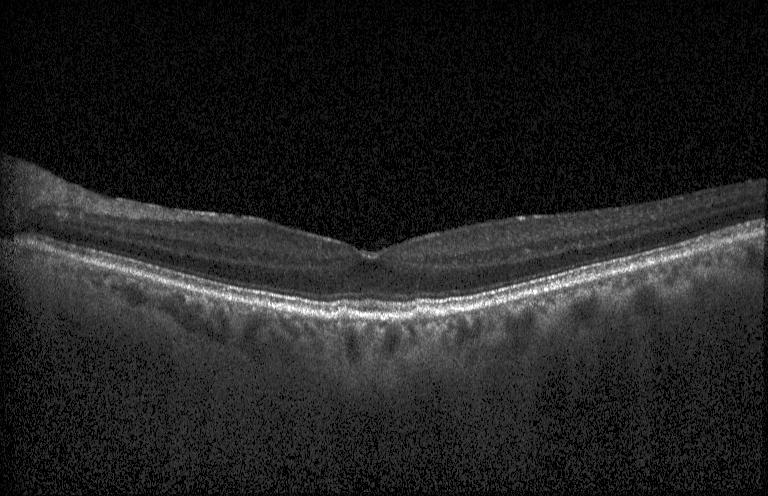 Sub-RPE drusenoid deposits.